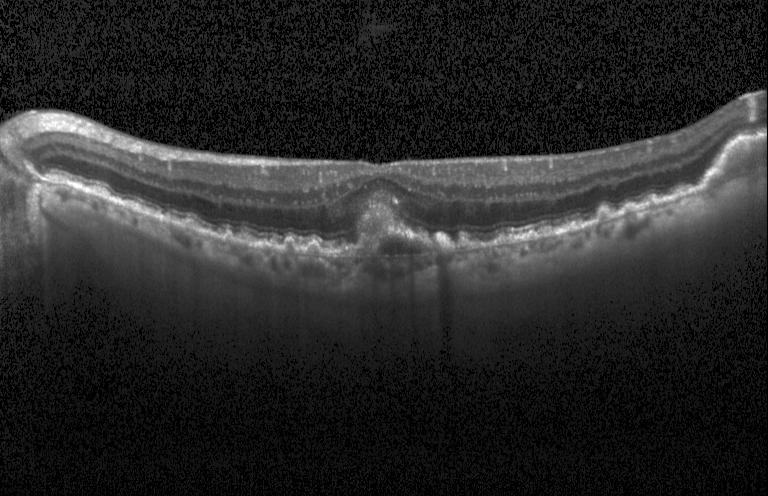
Finding: a choroidal neovascular membrane.